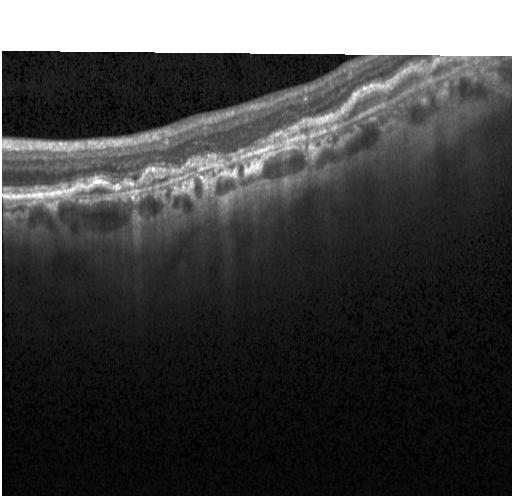
Retinal OCT cross-section — OCT finding: choroidal neovascularization (CNV).